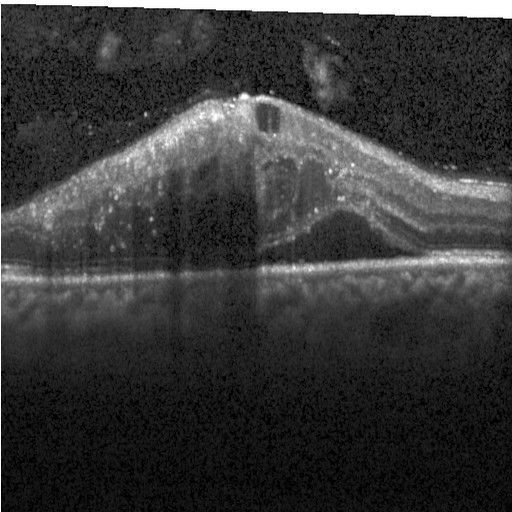

Fovea-centered. Acquired on a Heidelberg Spectralis. Optical coherence tomography B-scan. Spectral-domain optical coherence tomography
Impression: diabetic macular edema.